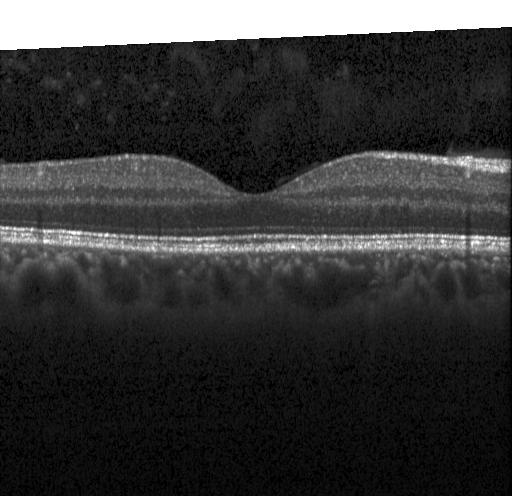
OCT B-scan, fovea-centered — Finding: no CNV, DME, or drusen.